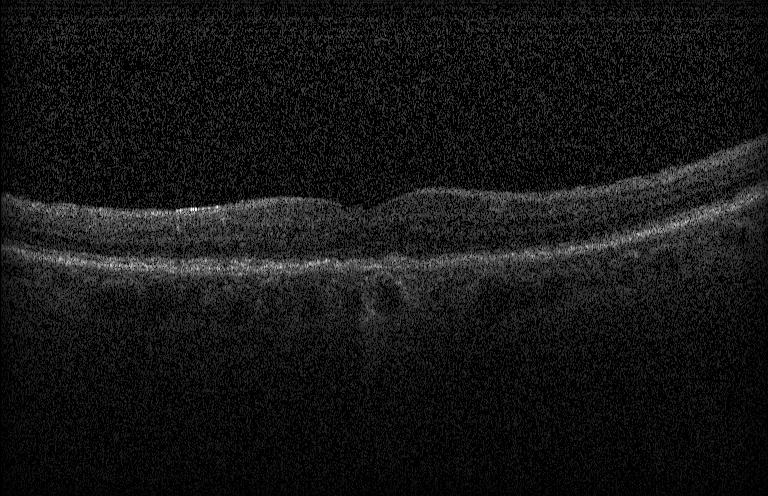

Dx: choroidal neovascularization (CNV).